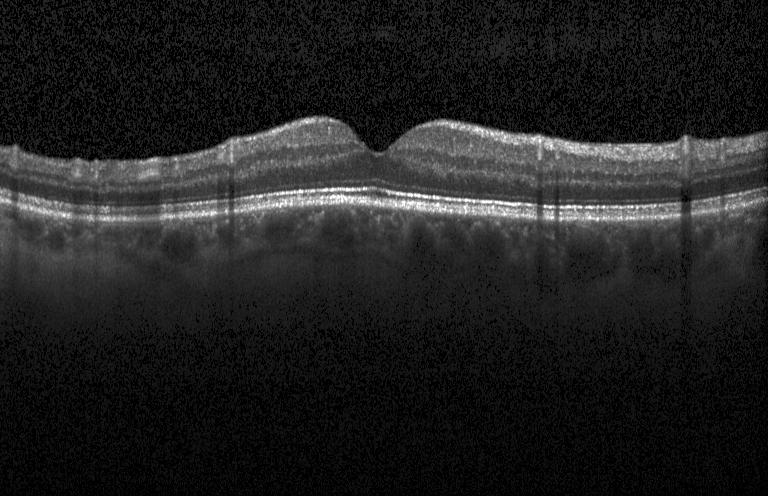
SD-OCT, OCT line scan, acquired on a Heidelberg Spectralis.
Diagnosis: no evidence of choroidal neovascularization, diabetic macular edema, or drusen.